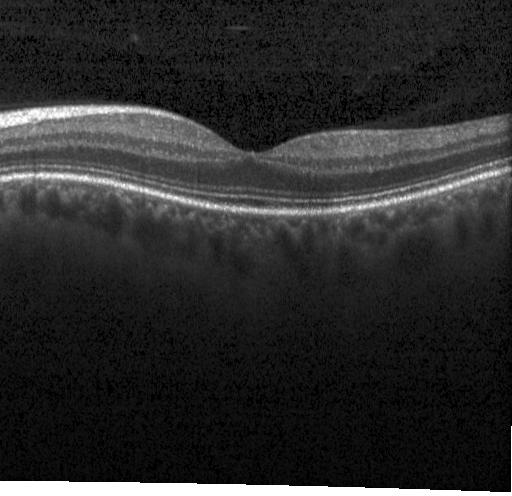
Diagnosis: no evidence of choroidal neovascularization, diabetic macular edema, or drusen.